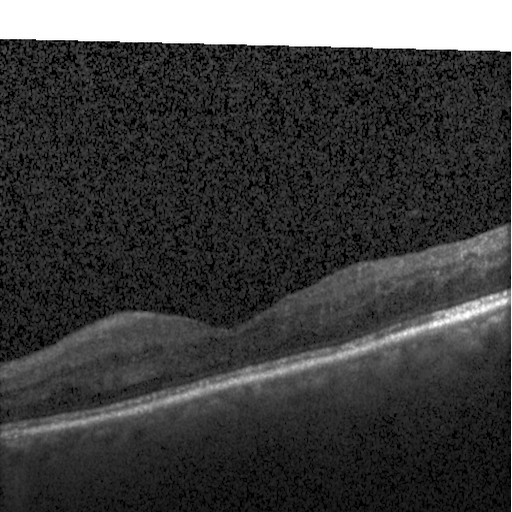 Fovea-centered. Optical coherence tomography scan
Diagnosis: diabetic macular edema.